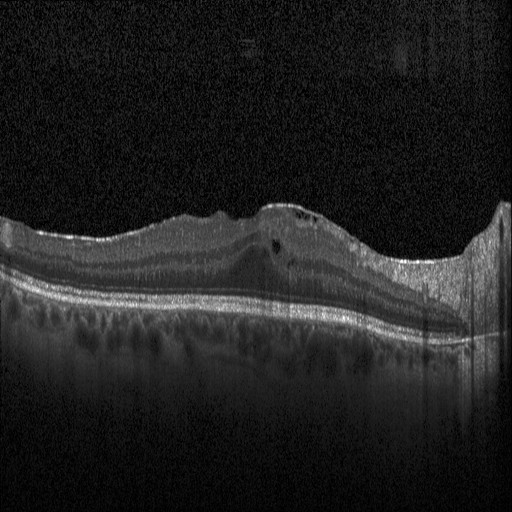 Optical coherence tomography scan; Heidelberg Spectralis OCT system — Diabetic macular edema (DME).